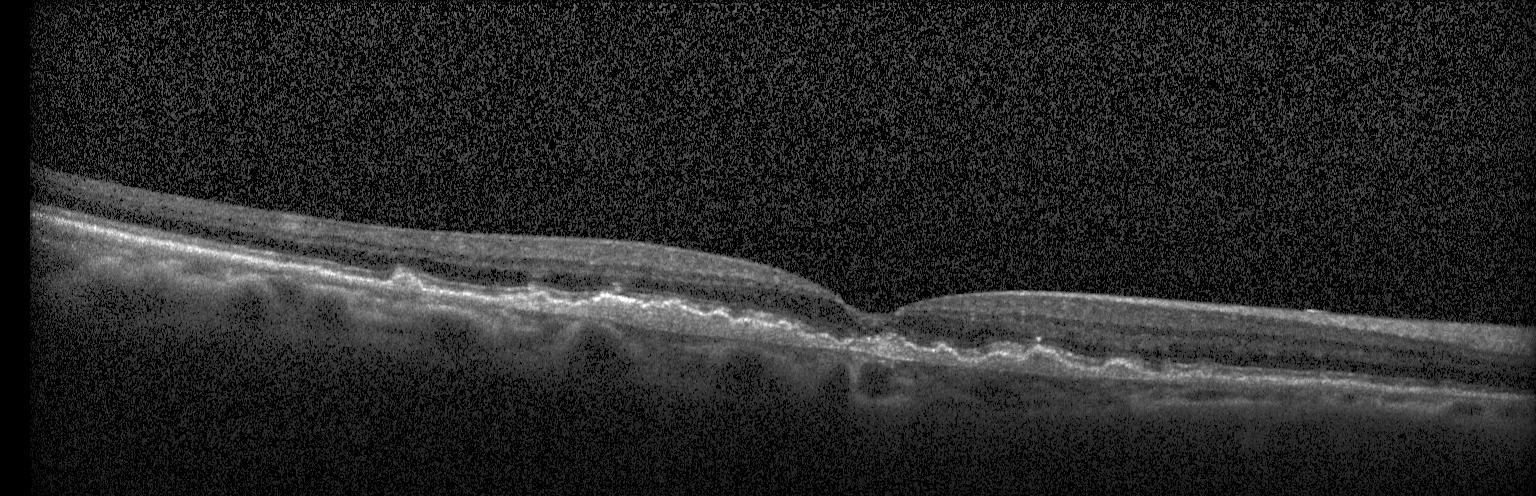

OCT B-scan · spectral-domain optical coherence tomography · acquired on a Heidelberg Spectralis. OCT finding: choroidal neovascularization.